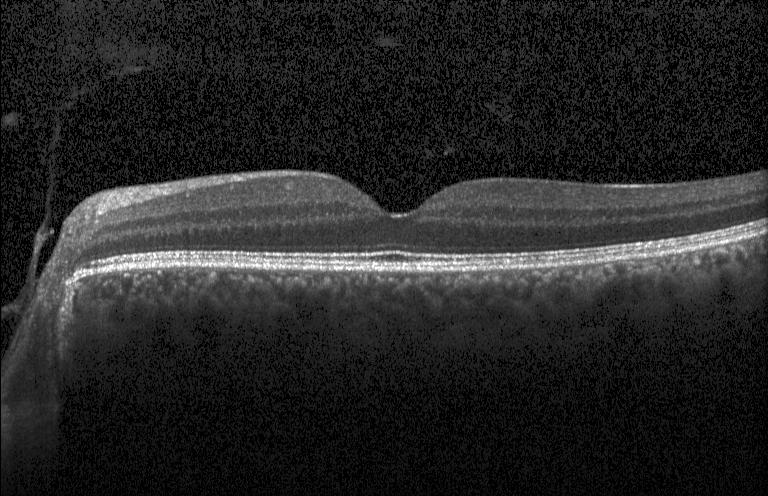 Spectral-domain OCT B-scan: no CNV, DME, or drusen.